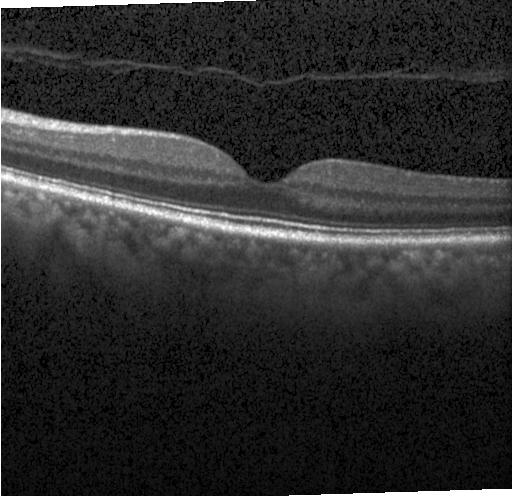

Acquired on a Heidelberg Spectralis. Optical coherence tomography scan.
Finding: no evidence of choroidal neovascularization, diabetic macular edema, or drusen.